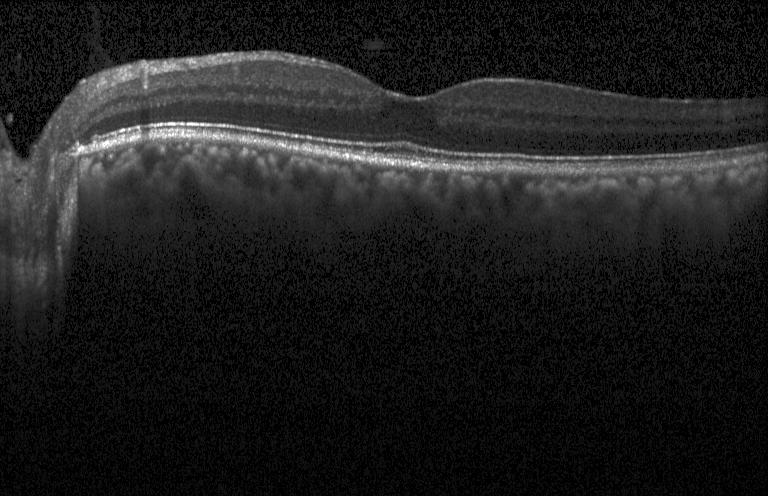

Optical coherence tomography scan.
Impression: neither choroidal neovascularization, diabetic macular edema, nor drusen.